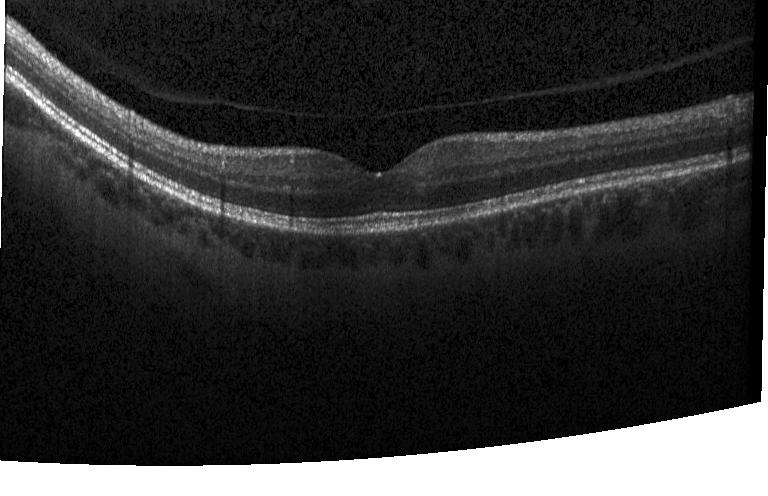

Heidelberg Spectralis; optical coherence tomography scan; spectral-domain OCT.
Macular OCT: no evidence of CNV, DME, or drusen.